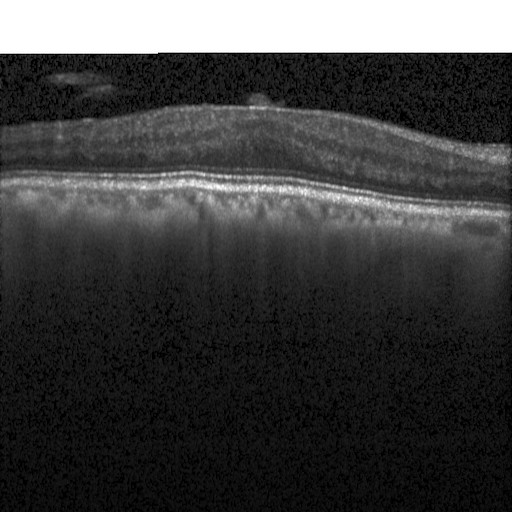
Heidelberg Spectralis OCT system · optical coherence tomography B-scan · macular scan.
This B-scan demonstrates diabetic macular edema (DME).